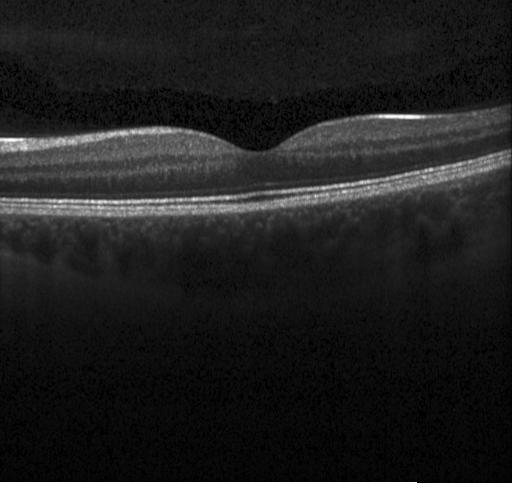
Optical coherence tomography scan
Impression: neither choroidal neovascularization, diabetic macular edema, nor drusen.